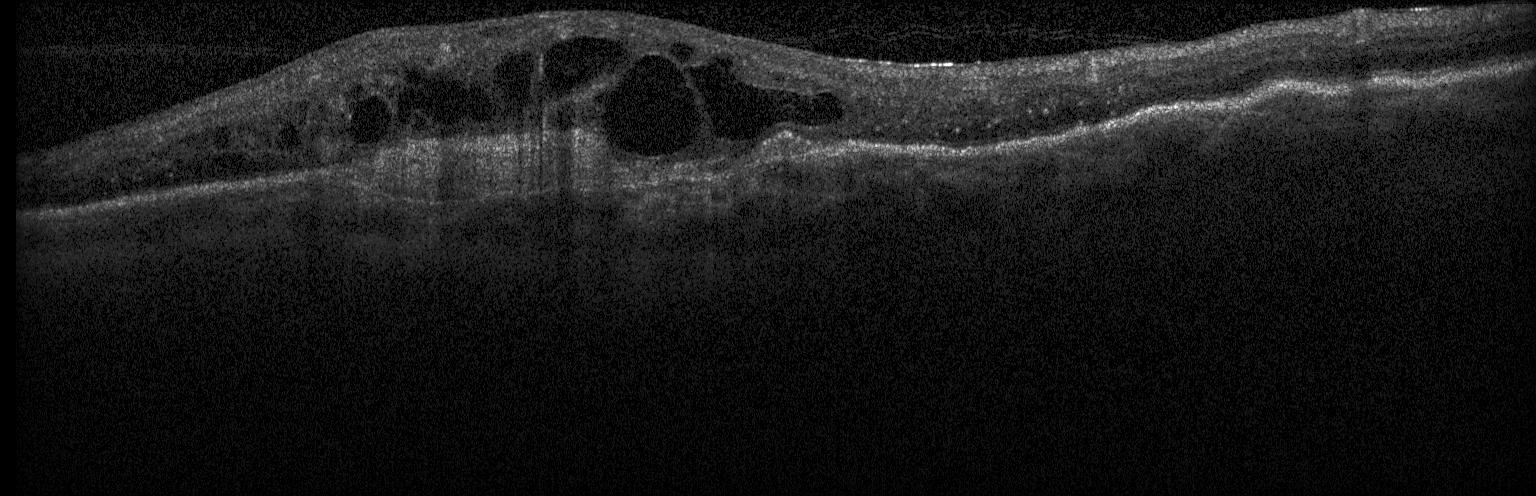 Retinal OCT B-scan, fovea-centered, Heidelberg Spectralis OCT system
Diagnosis: CNV.